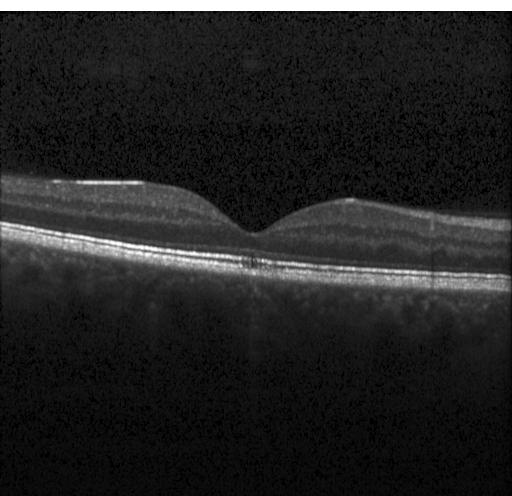 Diagnosis: neither CNV, DME, nor drusen.